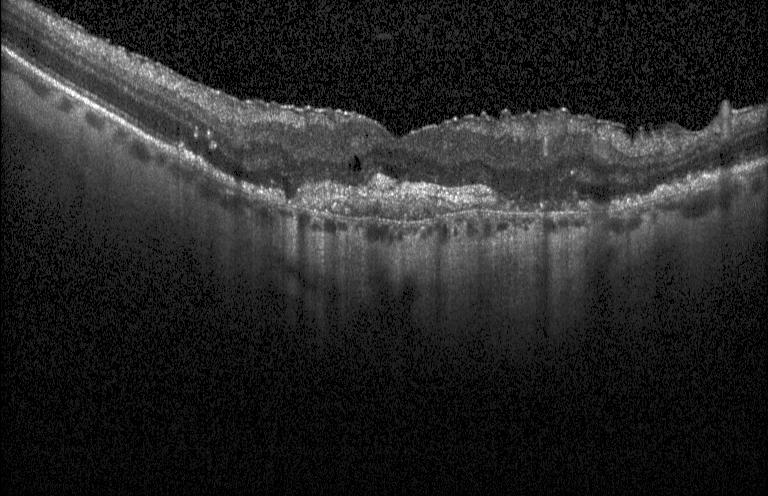 Macular OCT: CNV.